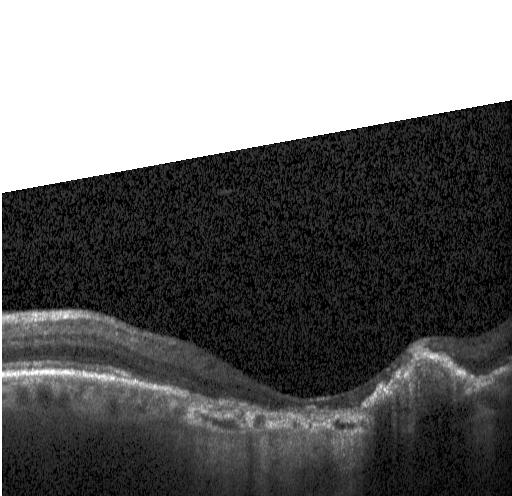 Optical coherence tomography scan
A choroidal neovascular membrane.